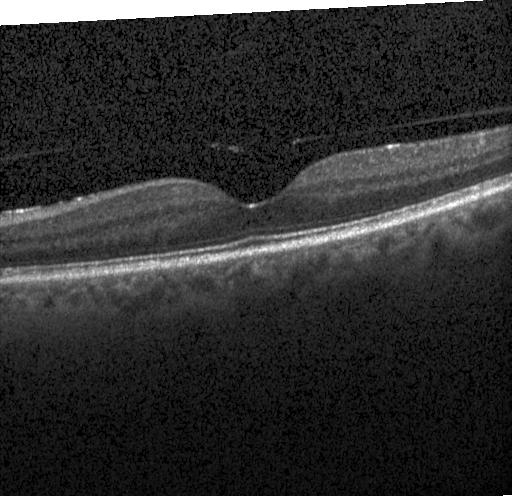
Centered on the fovea · optical coherence tomography scan · instrument: Heidelberg Spectralis — Impression: neither CNV, DME, nor drusen.